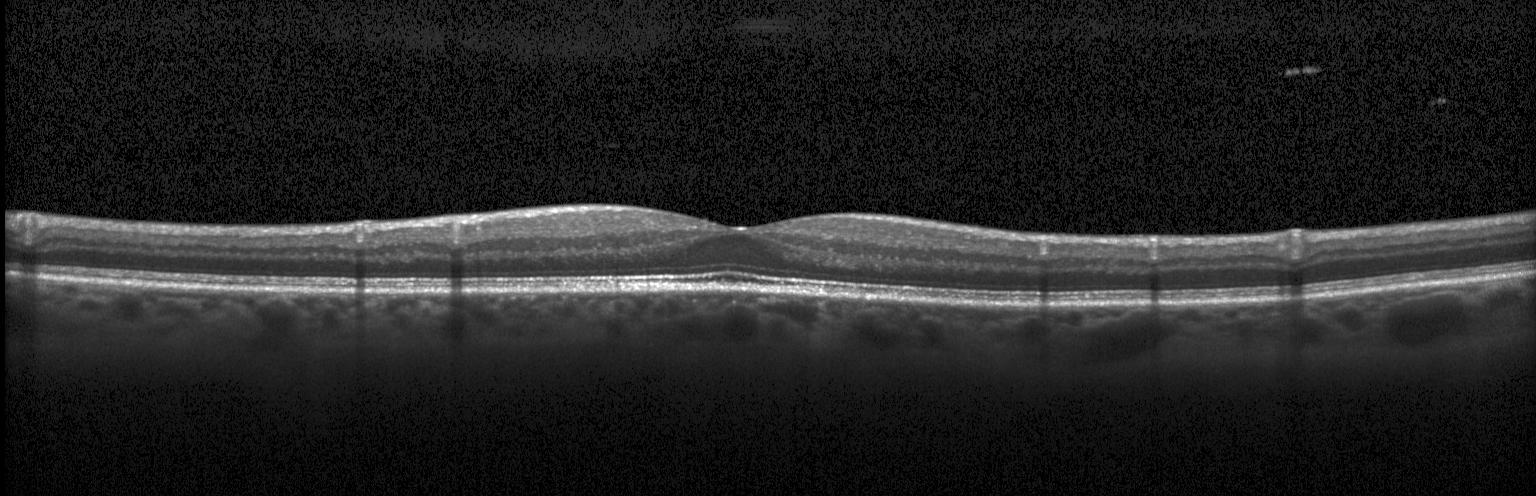
Horizontal scan through the fovea · retinal OCT cross-section · acquired on a Heidelberg Spectralis · spectral-domain optical coherence tomography — The scan shows no choroidal neovascularization, no diabetic macular edema, and no drusen.